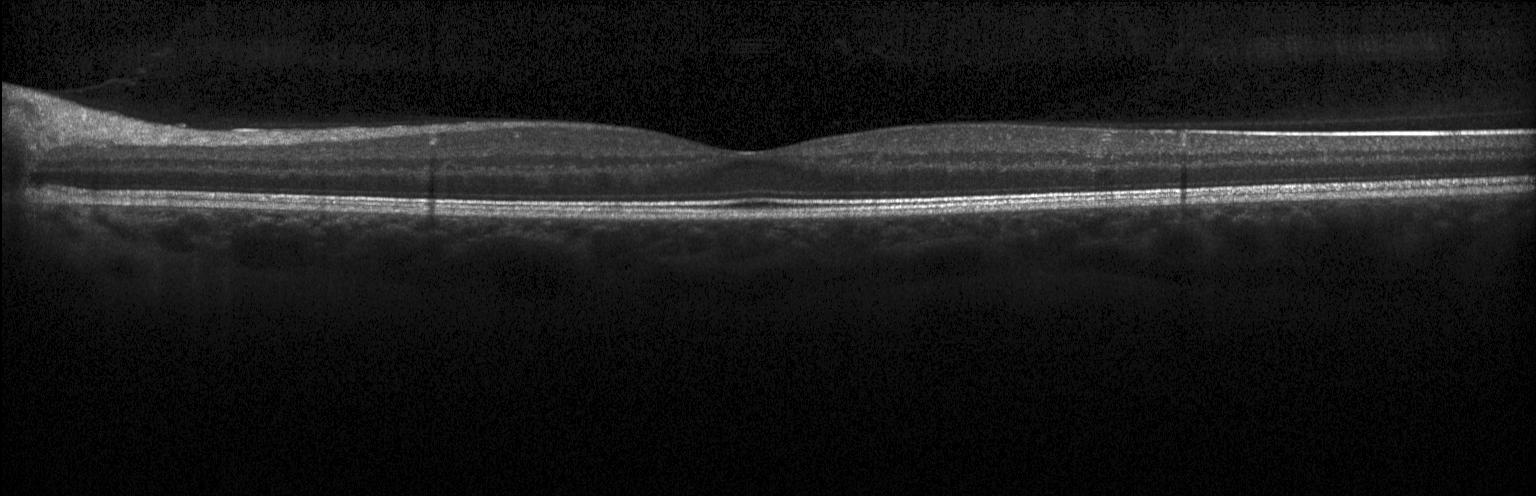 Assessment: neither choroidal neovascularization, diabetic macular edema, nor drusen.